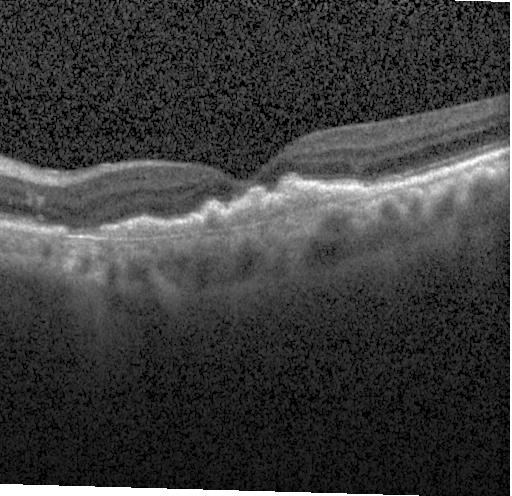

Diagnosis: a choroidal neovascular membrane.